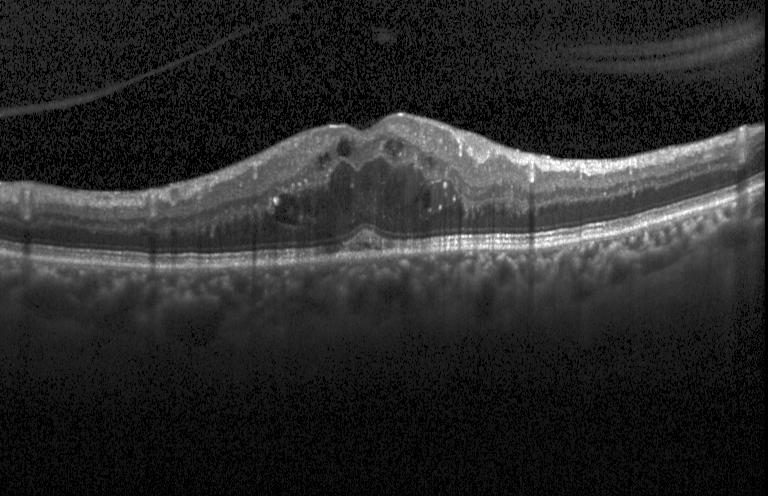 Optical coherence tomography B-scan.
Finding: diabetic macular edema.